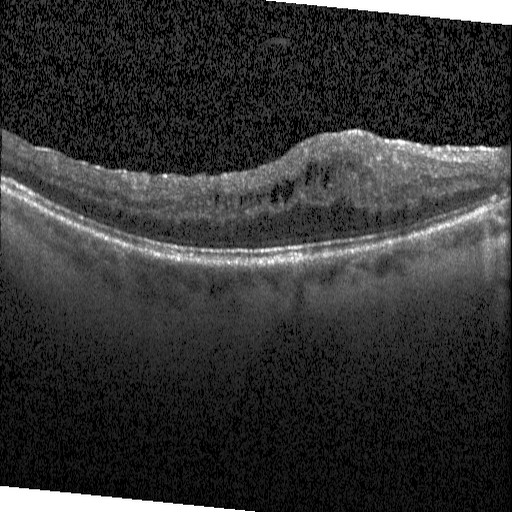 Spectral-domain OCT B-scan: diabetic macular edema.